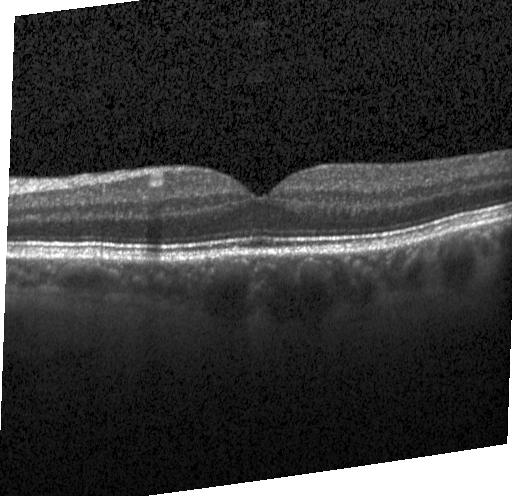

OCT B-scan — Finding: no evidence of choroidal neovascularization, diabetic macular edema, or drusen.